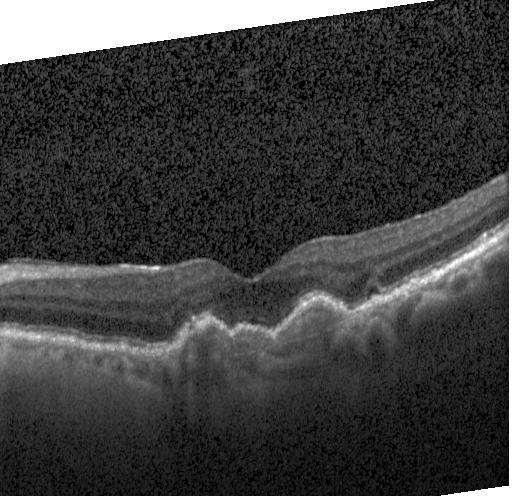
SD-OCT. Through the macula. Heidelberg Spectralis. Optical coherence tomography scan.
CNV.